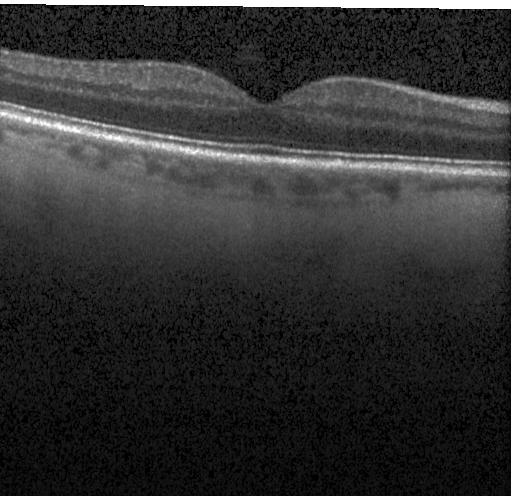 Spectral-domain OCT, Heidelberg Spectralis, retinal OCT cross-section, through the macula
Assessment: no CNV, no DME, and no drusen.